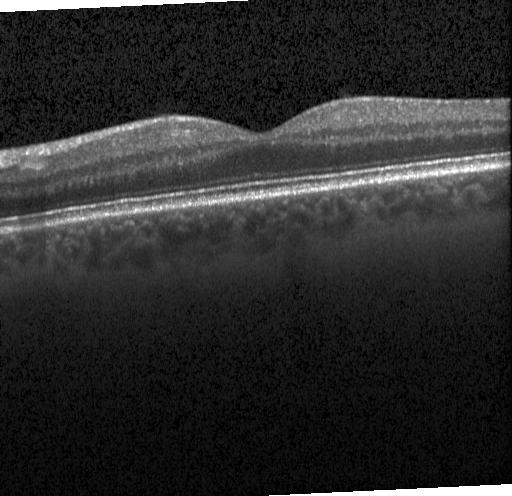 OCT B-scan; centered on the fovea; instrument: Heidelberg Spectralis. No choroidal neovascularization, diabetic macular edema, or drusen.